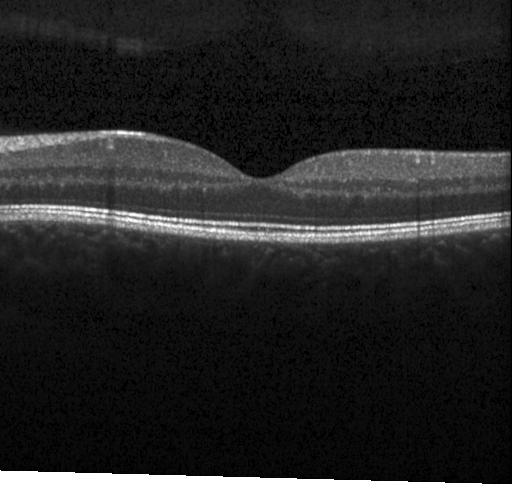

Retinal OCT cross-section
Macular OCT: no evidence of choroidal neovascularization, diabetic macular edema, or drusen.